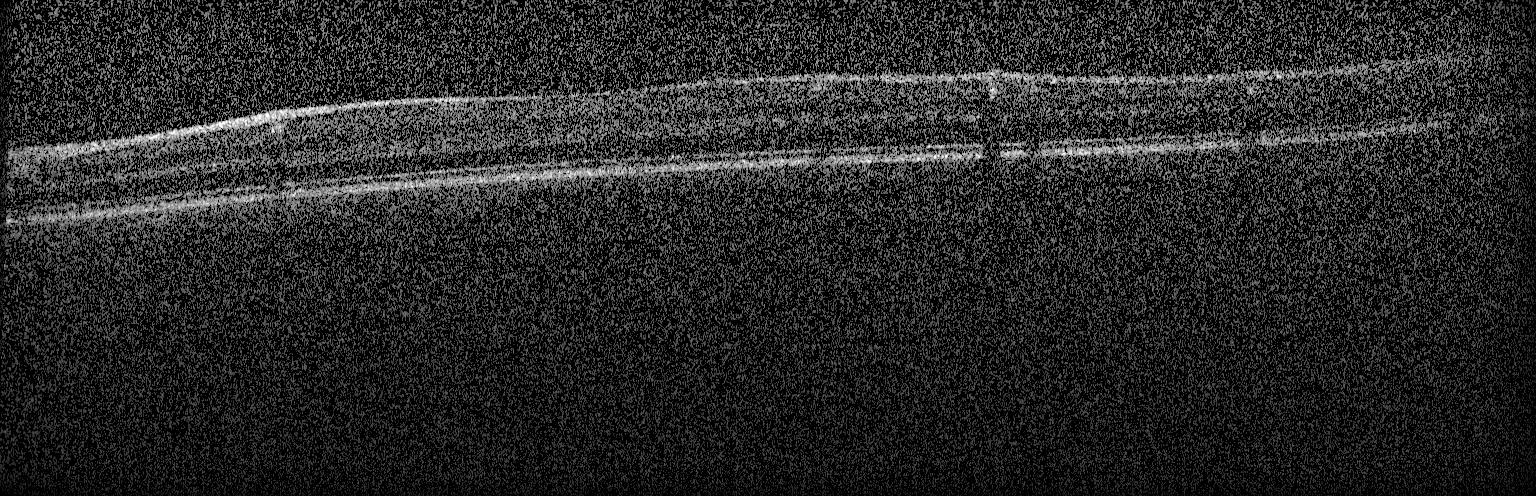
Heidelberg Spectralis OCT system; fovea-centered; spectral-domain OCT; retinal OCT cross-section.
The scan shows no choroidal neovascularization, no diabetic macular edema, and no drusen.